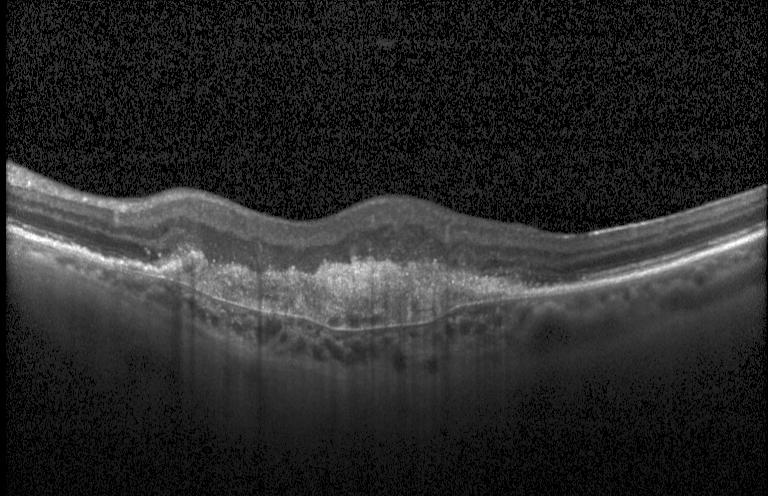

Optical coherence tomography scan. Heidelberg Spectralis.
Finding: a choroidal neovascular membrane.